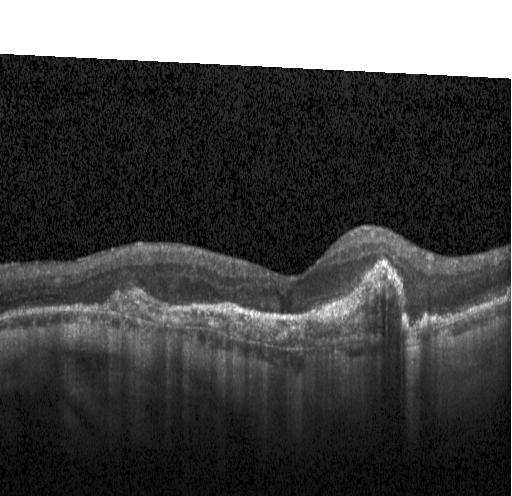 Impression: a choroidal neovascular membrane.